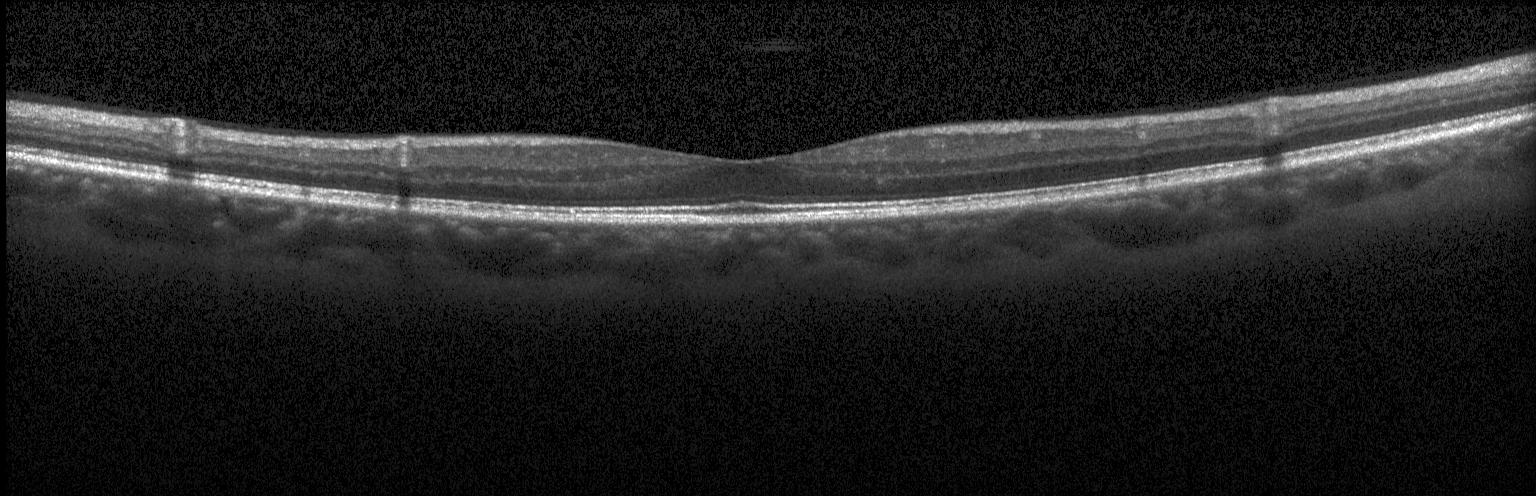
Retinal OCT B-scan; acquired on a Heidelberg Spectralis; SD-OCT
Impression: no CNV, no DME, and no drusen.